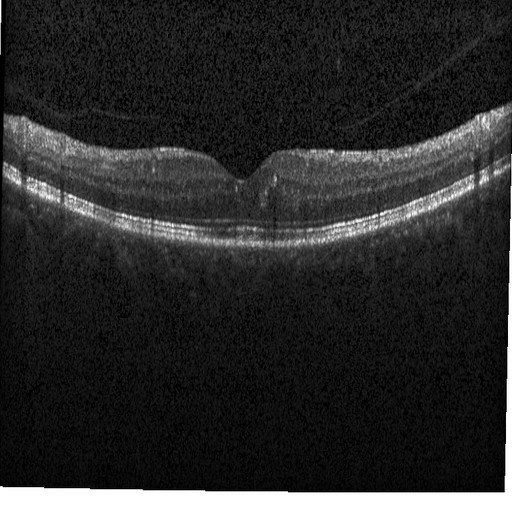 Retinal OCT cross-section — The scan shows diabetic macular edema (DME).